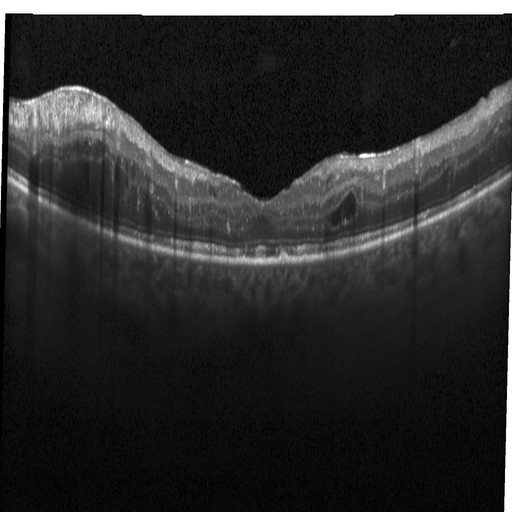

OCT line scan · spectral-domain OCT. DME.